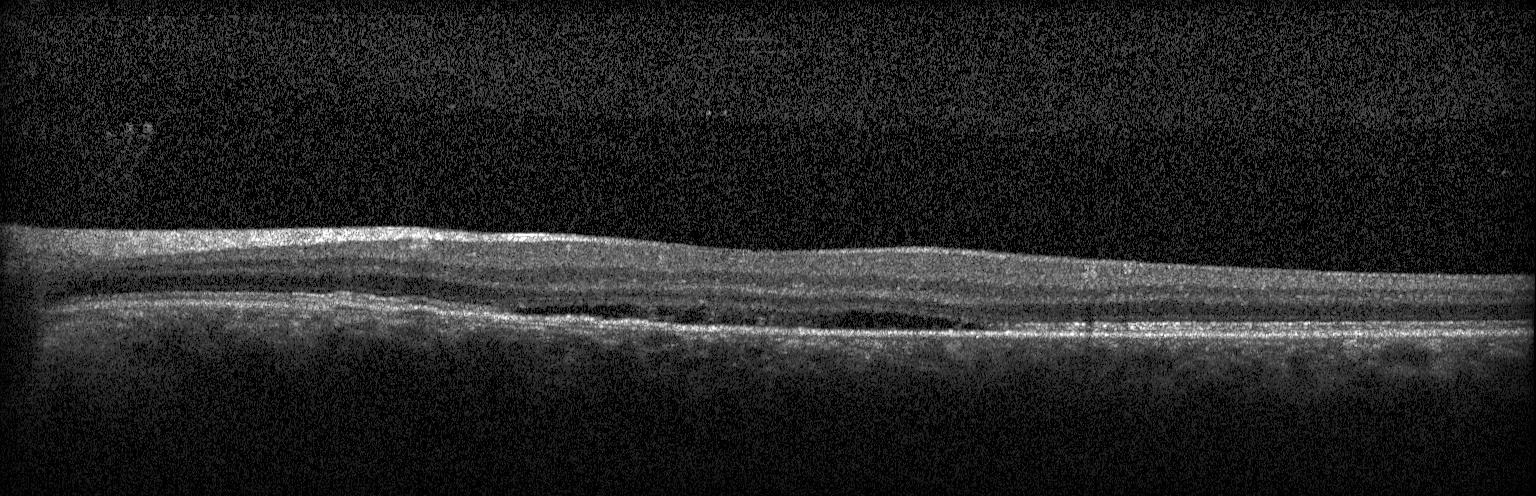

Fovea-centered; spectral-domain optical coherence tomography; optical coherence tomography scan
Impression: a choroidal neovascular membrane.